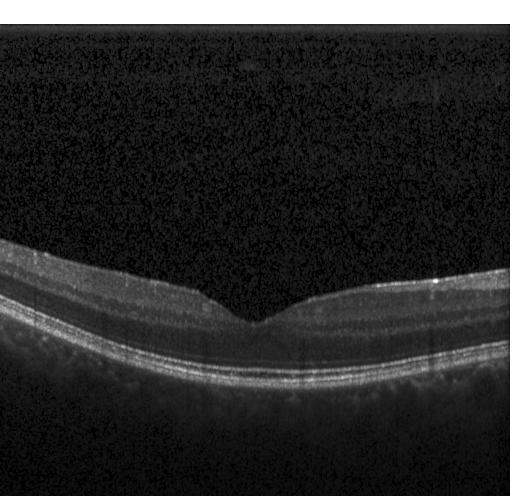

OCT B-scan · spectral-domain OCT · centered on the fovea — Finding: no CNV, no DME, and no drusen.